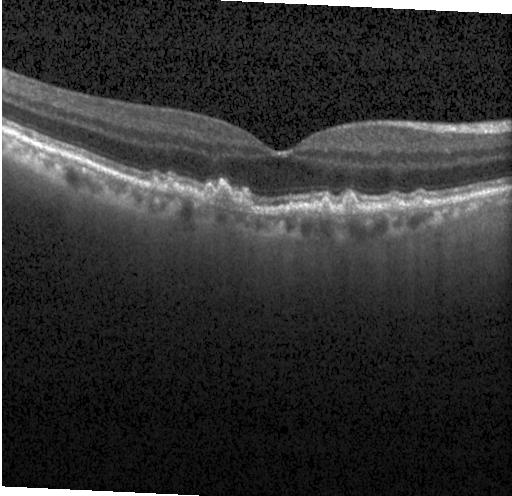

Optical coherence tomography scan; SD-OCT; centered on the fovea; Heidelberg Spectralis OCT system. This B-scan demonstrates sub-RPE drusenoid deposits.